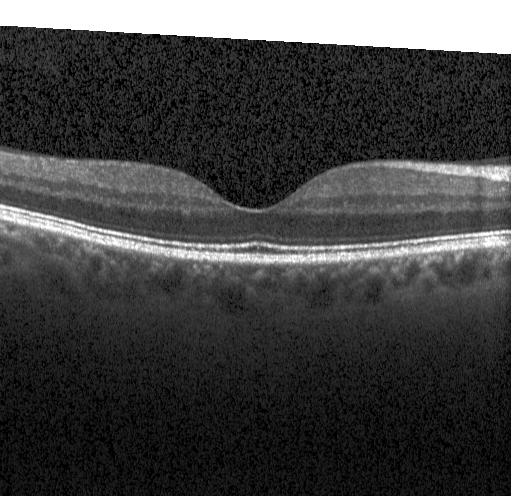 Impression: no CNV, no DME, and no drusen.